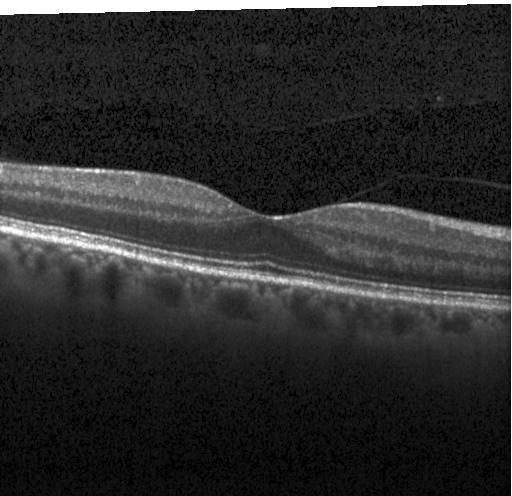

Retinal OCT B-scan; instrument: Heidelberg Spectralis.
Assessment: no choroidal neovascularization, diabetic macular edema, or drusen.